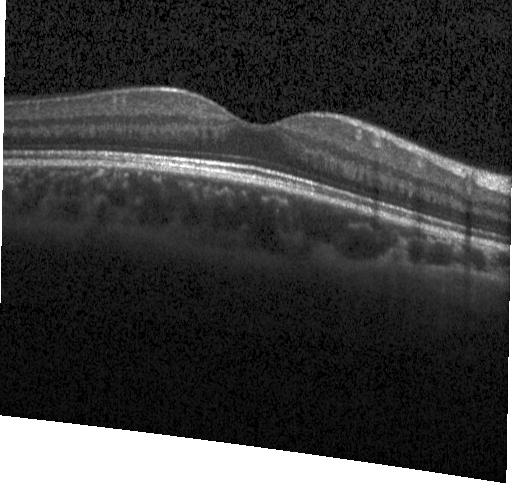

Instrument: Heidelberg Spectralis. OCT B-scan
Impression: no CNV, DME, or drusen.